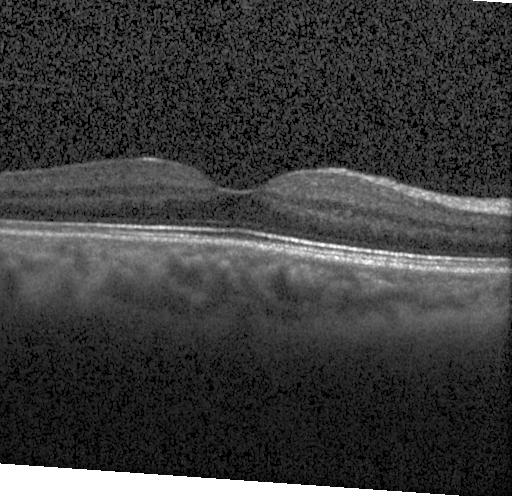

Macular OCT: no evidence of CNV, DME, or drusen.